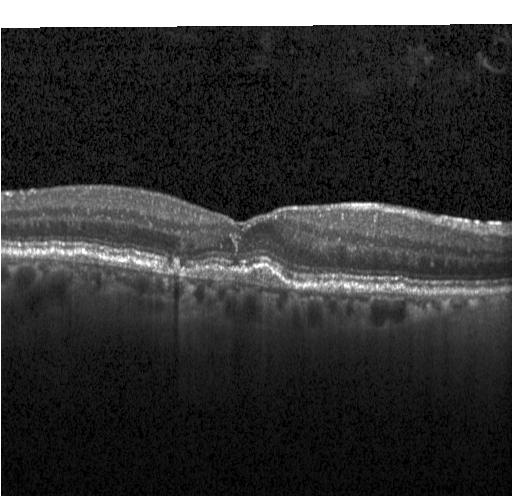

Assessment: CNV.